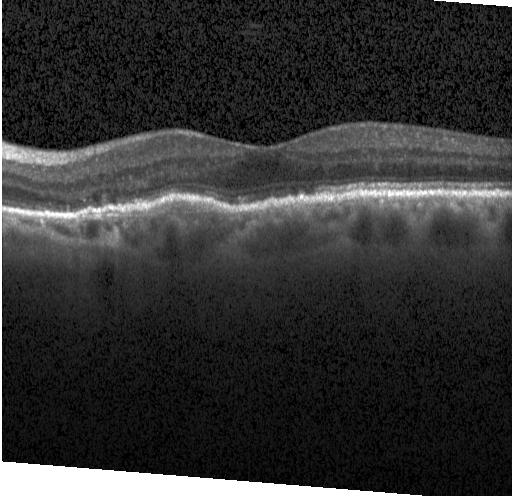 Retinal OCT cross-section.
A choroidal neovascular membrane.